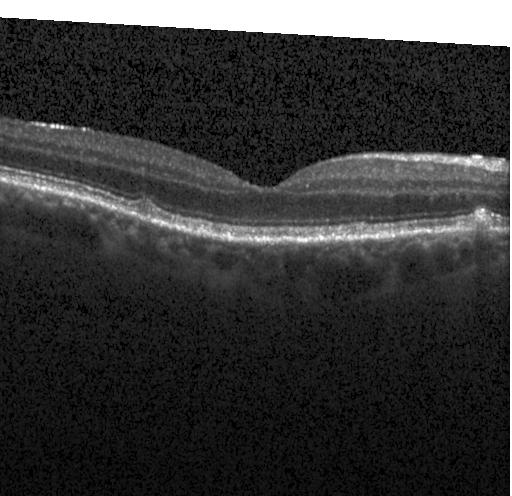
OCT line scan · spectral-domain OCT. Sub-RPE drusenoid deposits.